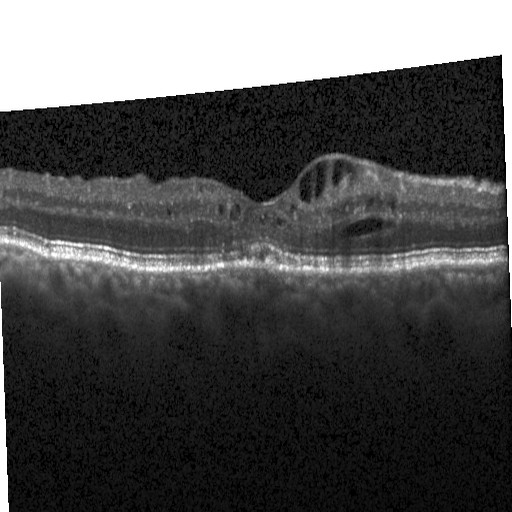 Spectral-domain OCT; instrument: Heidelberg Spectralis; OCT line scan. Finding: diabetic macular edema.